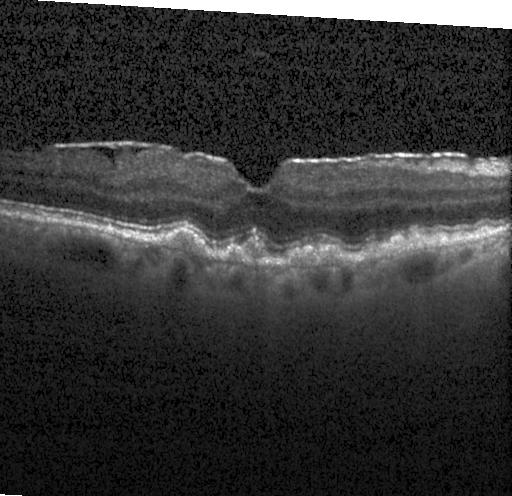
Finding: drusen.